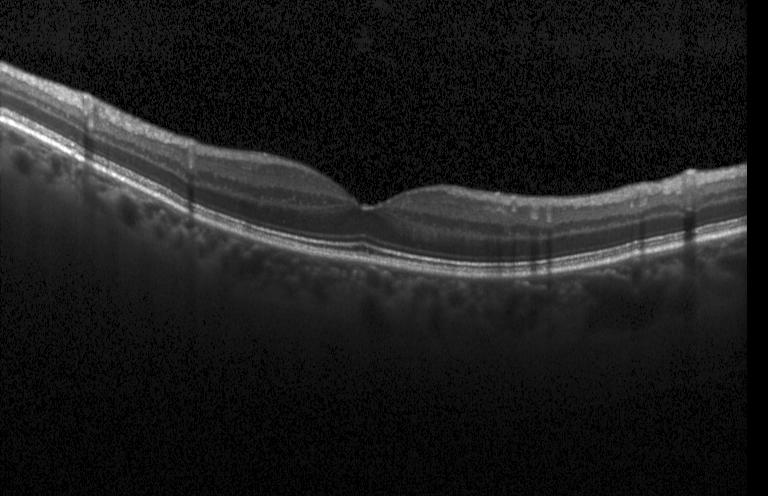
OCT finding: neither choroidal neovascularization, diabetic macular edema, nor drusen.